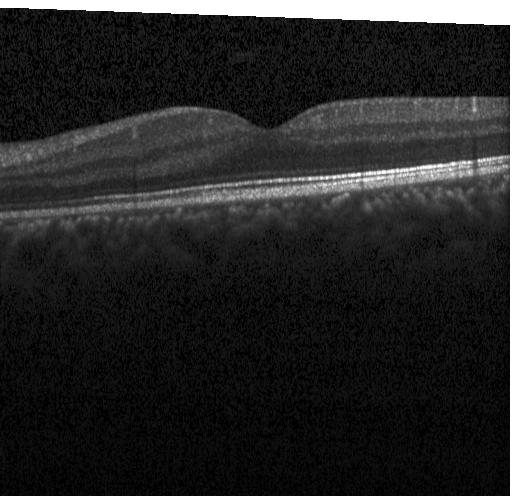

Fovea-centered; OCT B-scan; instrument: Heidelberg Spectralis
Diagnosis: neither choroidal neovascularization, diabetic macular edema, nor drusen.